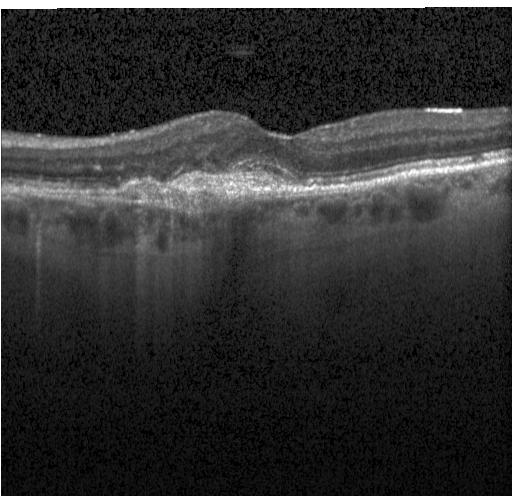 Retinal OCT B-scan. Finding: choroidal neovascularization.